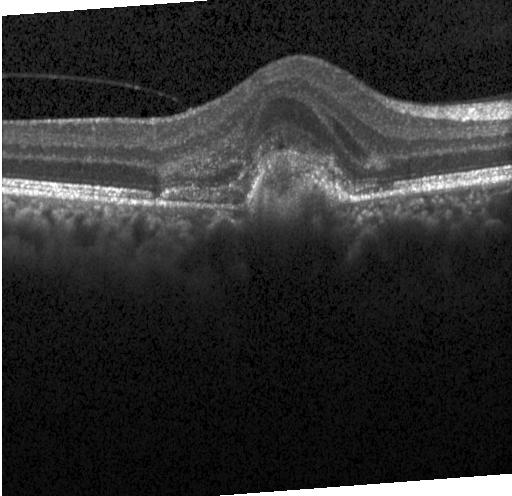

This B-scan demonstrates a choroidal neovascular membrane.